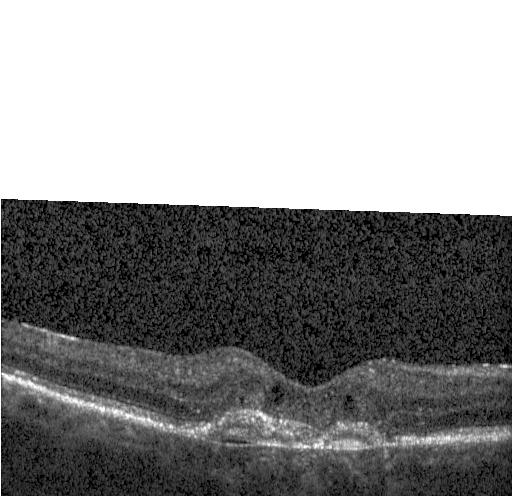
OCT line scan · Heidelberg Spectralis OCT system · SD-OCT · fovea-centered. Dx: choroidal neovascularization (CNV).